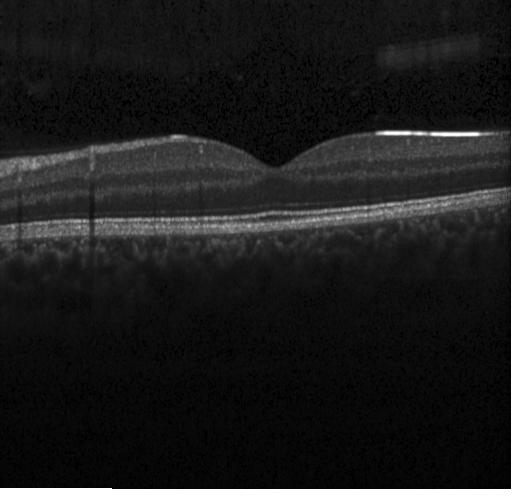
Retinal OCT cross-section; Heidelberg Spectralis OCT system. Macular OCT: no CNV, DME, or drusen.